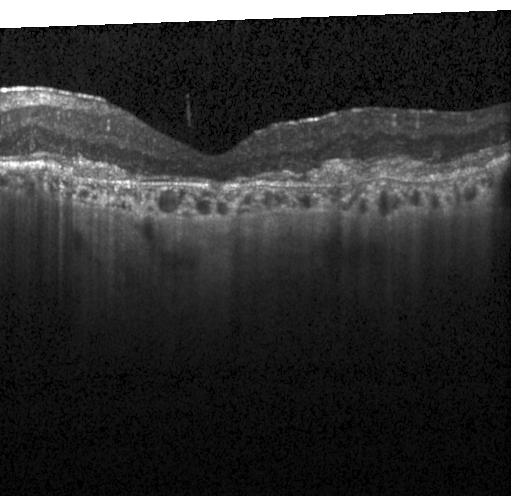
Heidelberg Spectralis OCT system · fovea-centered · SD-OCT · optical coherence tomography scan — Finding: a choroidal neovascular membrane.